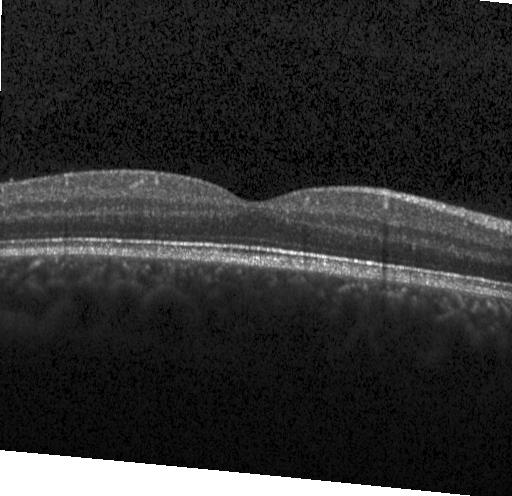
OCT scan showing no CNV, DME, or drusen.